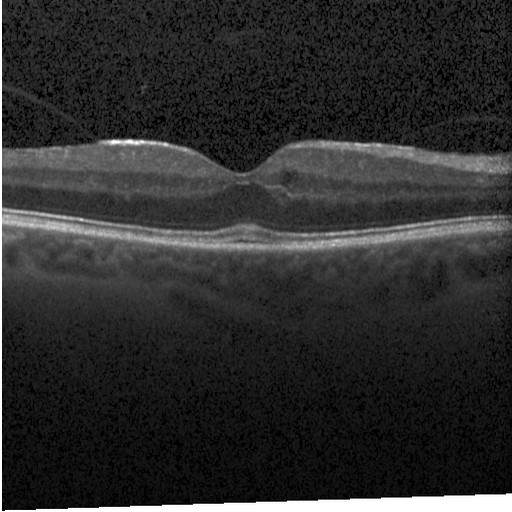 Retinal OCT cross-section showing diabetic macular edema.